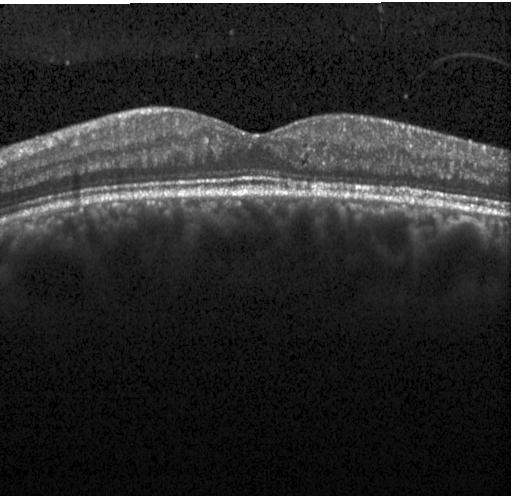

Through the macula · optical coherence tomography scan · acquired on a Heidelberg Spectralis · SD-OCT.
Diagnosis: no choroidal neovascularization, no diabetic macular edema, and no drusen.